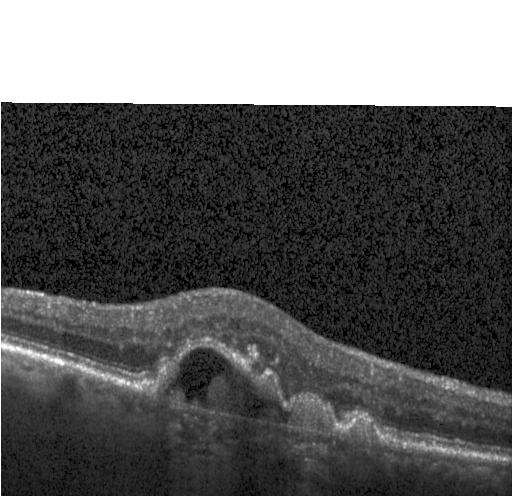

Retinal OCT B-scan. Macular scan. Impression: choroidal neovascularization.